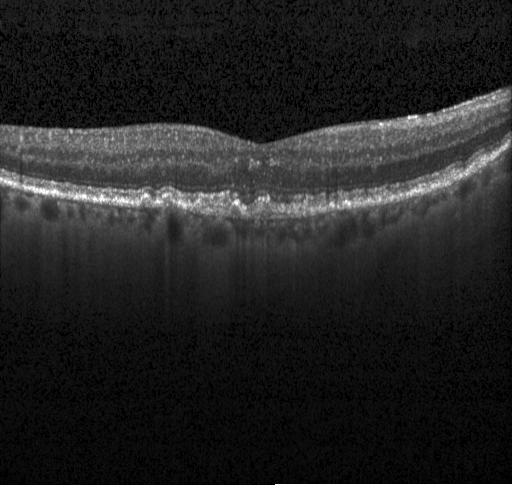
Retinal OCT B-scan. Heidelberg Spectralis OCT system. SD-OCT. Centered on the fovea — Impression: drusen.